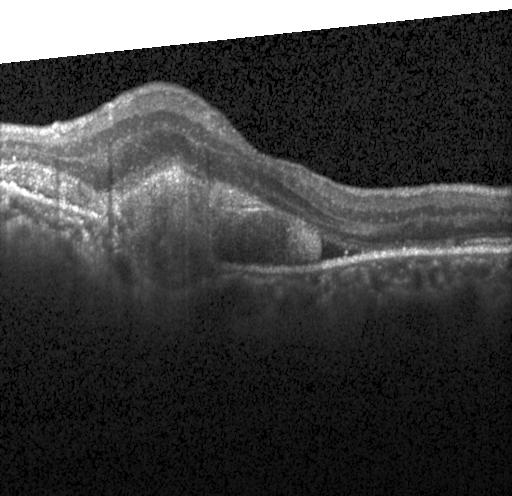

Macular OCT demonstrating choroidal neovascularization (CNV).